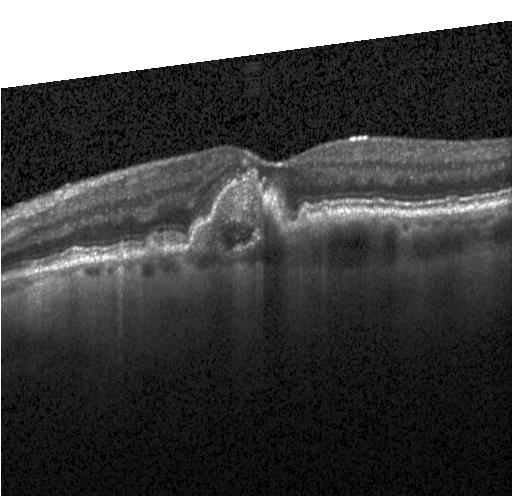 Spectral-domain OCT, optical coherence tomography scan, instrument: Heidelberg Spectralis.
Impression: choroidal neovascularization.